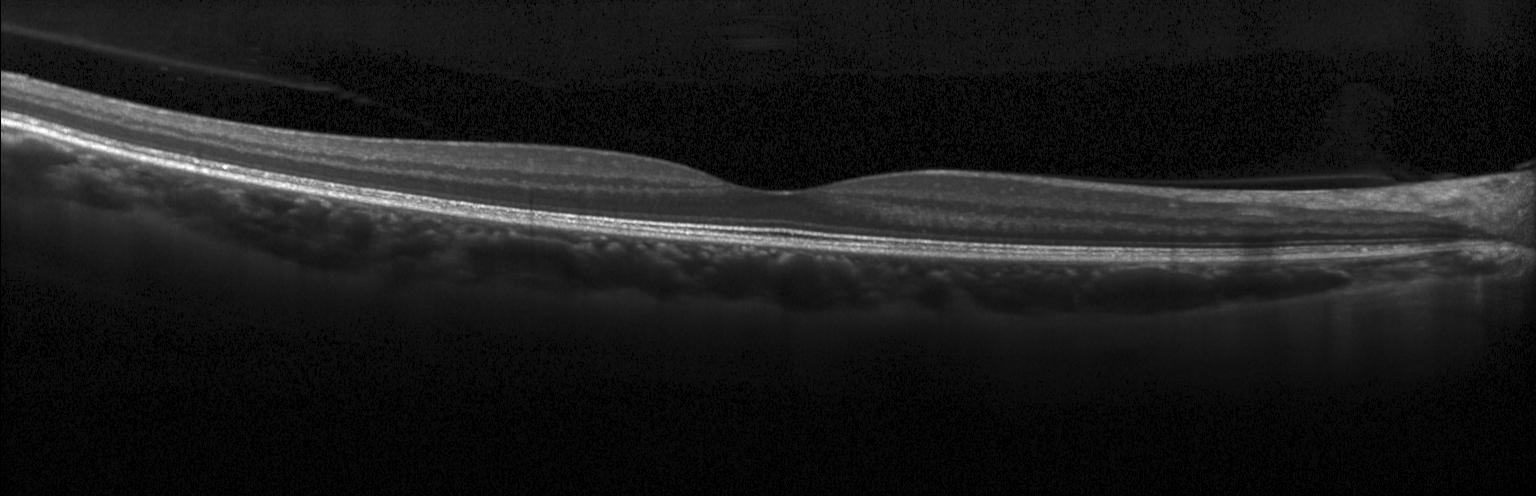 OCT line scan · SD-OCT
Impression: neither choroidal neovascularization, diabetic macular edema, nor drusen.